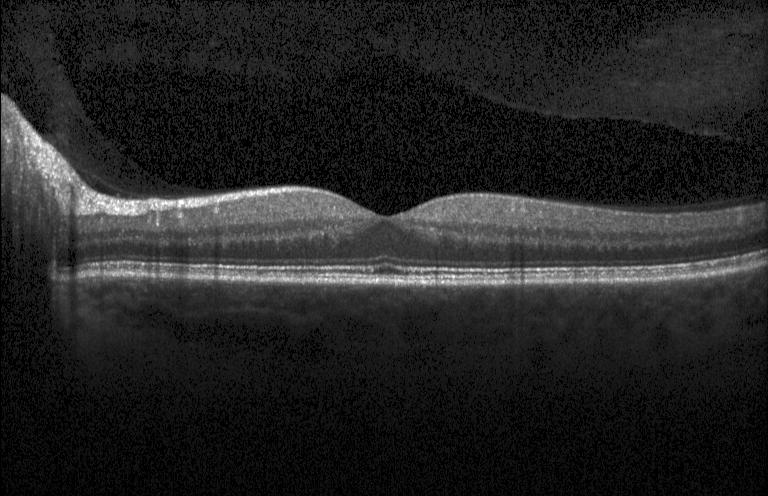
Heidelberg Spectralis; centered on the fovea; spectral-domain OCT; retinal OCT B-scan — No choroidal neovascularization, no diabetic macular edema, and no drusen.